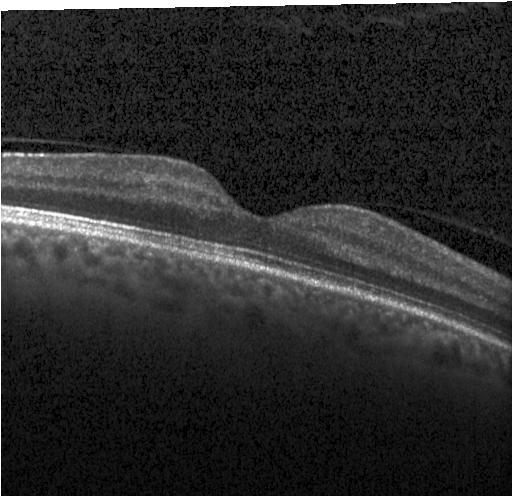

Finding: neither CNV, DME, nor drusen.